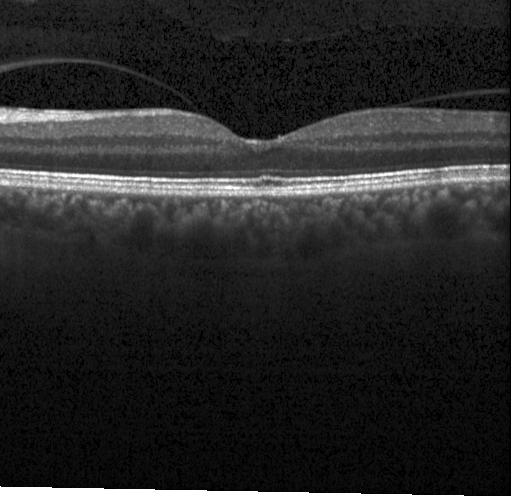
Optical coherence tomography B-scan
Impression: no evidence of choroidal neovascularization, diabetic macular edema, or drusen.